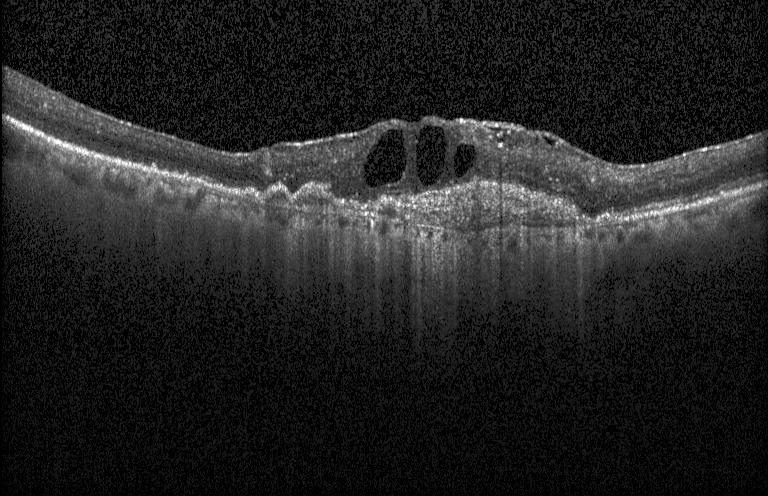

Spectral-domain OCT; optical coherence tomography scan. Finding: choroidal neovascularization.